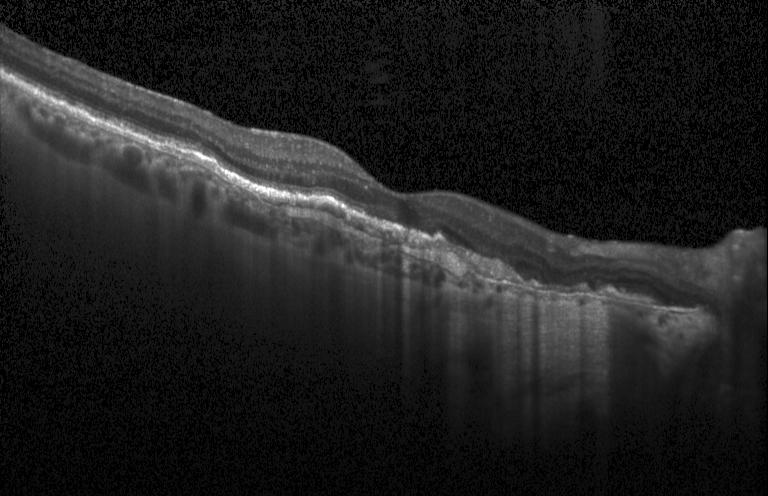

Spectral-domain OCT B-scan: choroidal neovascularization (CNV).